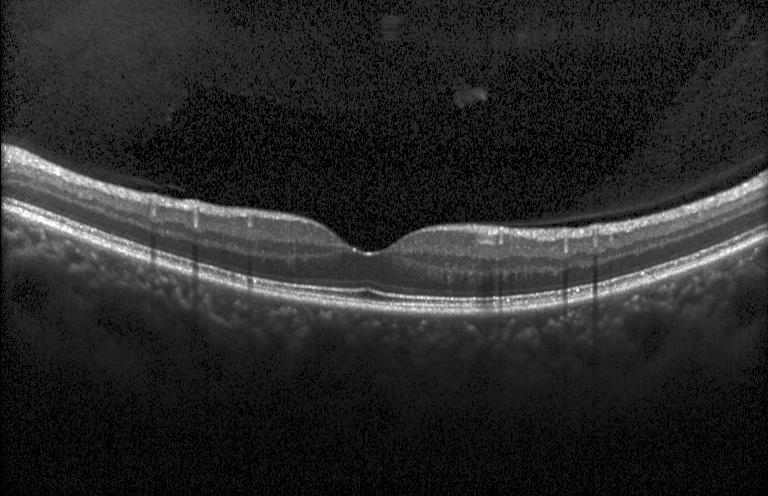

Impression: no choroidal neovascularization, diabetic macular edema, or drusen.